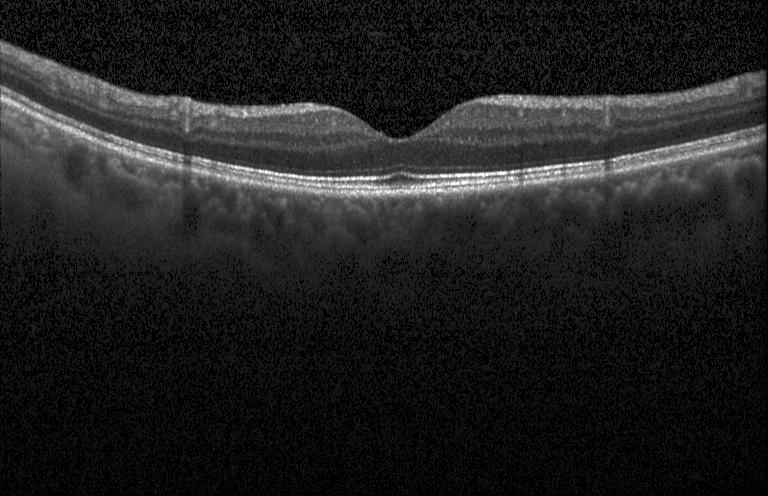
OCT scan showing no evidence of choroidal neovascularization, diabetic macular edema, or drusen.